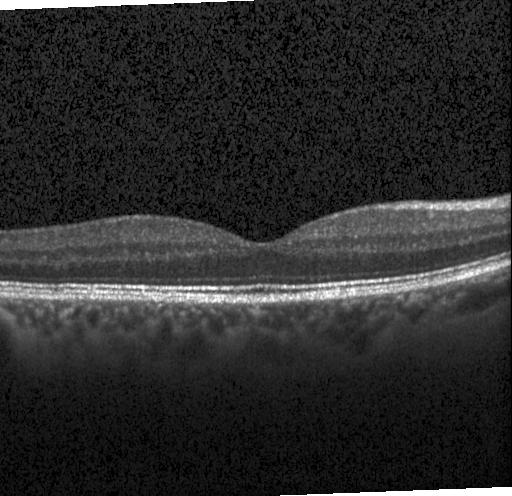

Retinal OCT B-scan. Diagnosis: no choroidal neovascularization, no diabetic macular edema, and no drusen.